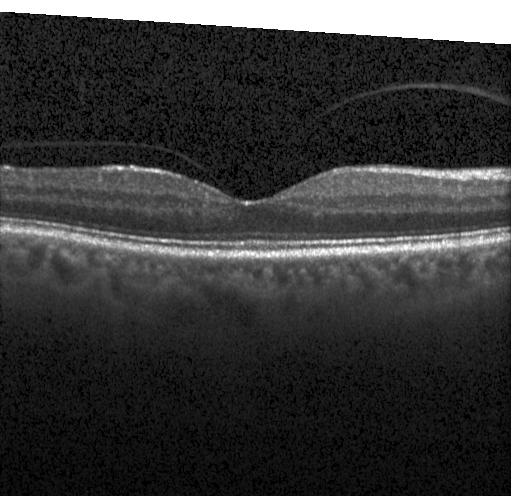
Horizontal scan through the fovea; retinal OCT cross-section
This B-scan demonstrates no evidence of choroidal neovascularization, diabetic macular edema, or drusen.